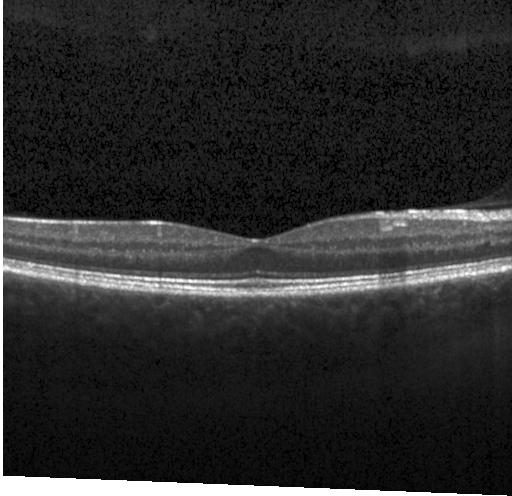 No evidence of CNV, DME, or drusen.